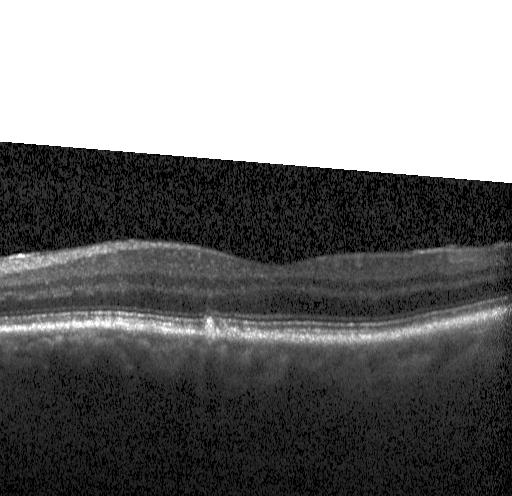 Optical coherence tomography B-scan — Diagnosis: sub-RPE drusenoid deposits.